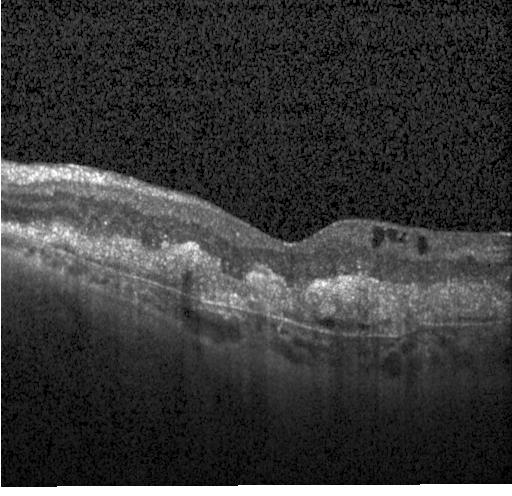

Macular OCT: a choroidal neovascular membrane.